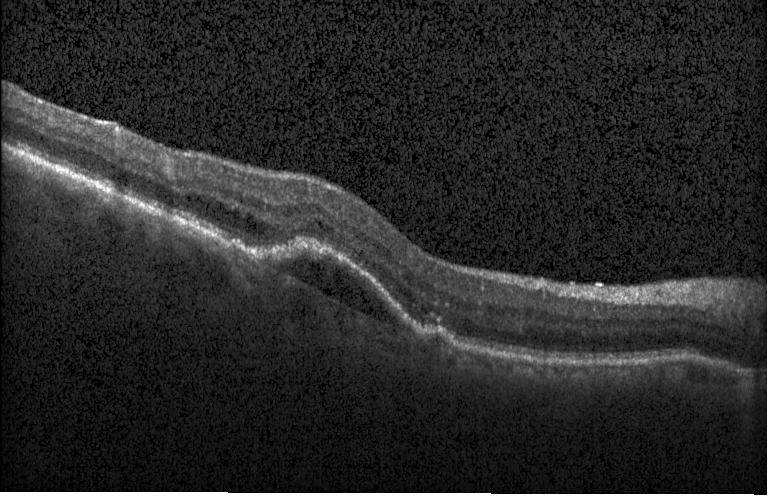

Fovea-centered · spectral-domain OCT · OCT B-scan · acquired on a Heidelberg Spectralis
Impression: CNV.